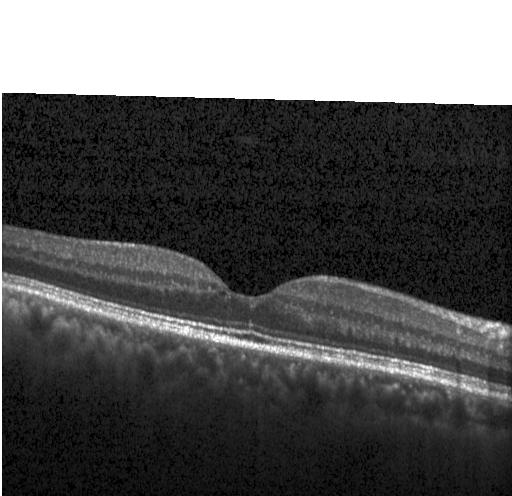 This B-scan demonstrates no choroidal neovascularization, diabetic macular edema, or drusen.